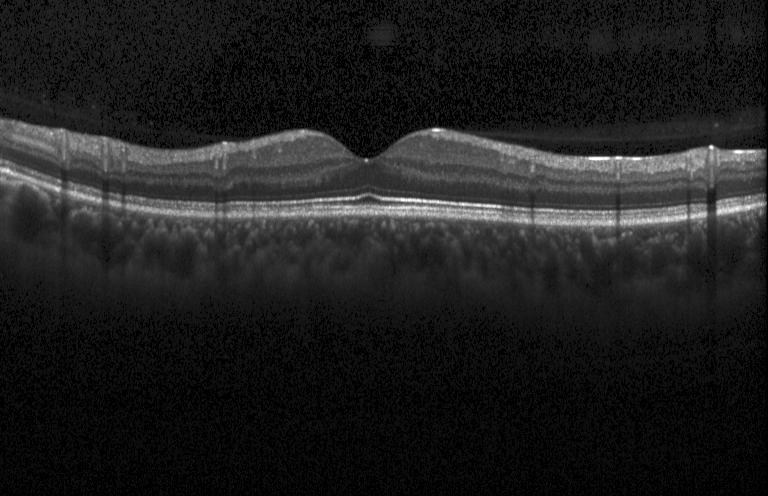 The scan shows no evidence of CNV, DME, or drusen.